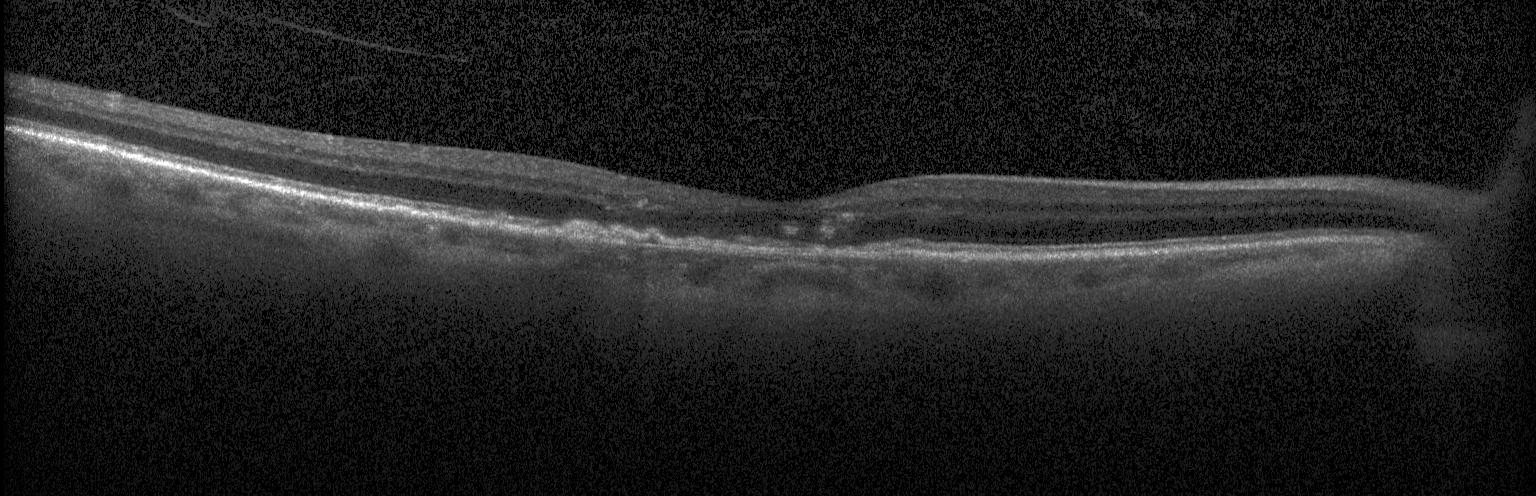 Retinal OCT B-scan, spectral-domain optical coherence tomography, macular scan — Macular OCT: choroidal neovascularization (CNV).